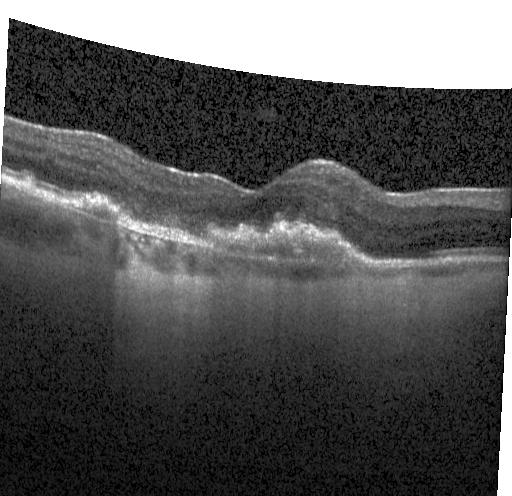 Finding: choroidal neovascularization.